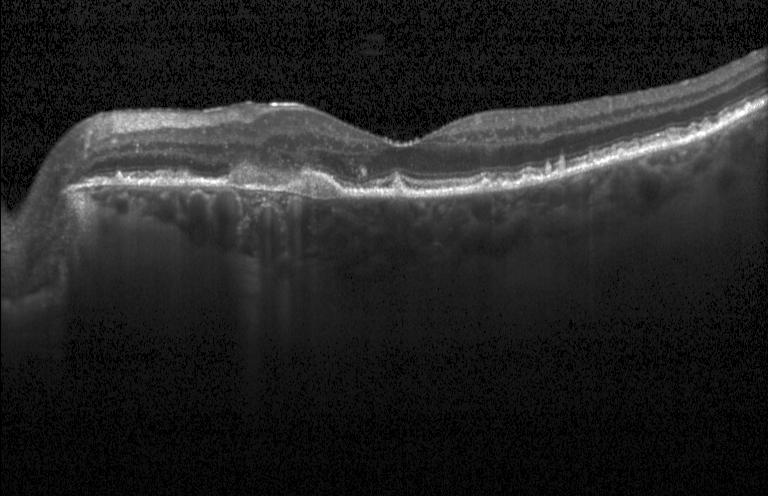

Instrument: Heidelberg Spectralis. Macular scan. Retinal OCT B-scan. Spectral-domain optical coherence tomography — Diagnosis: choroidal neovascularization (CNV).